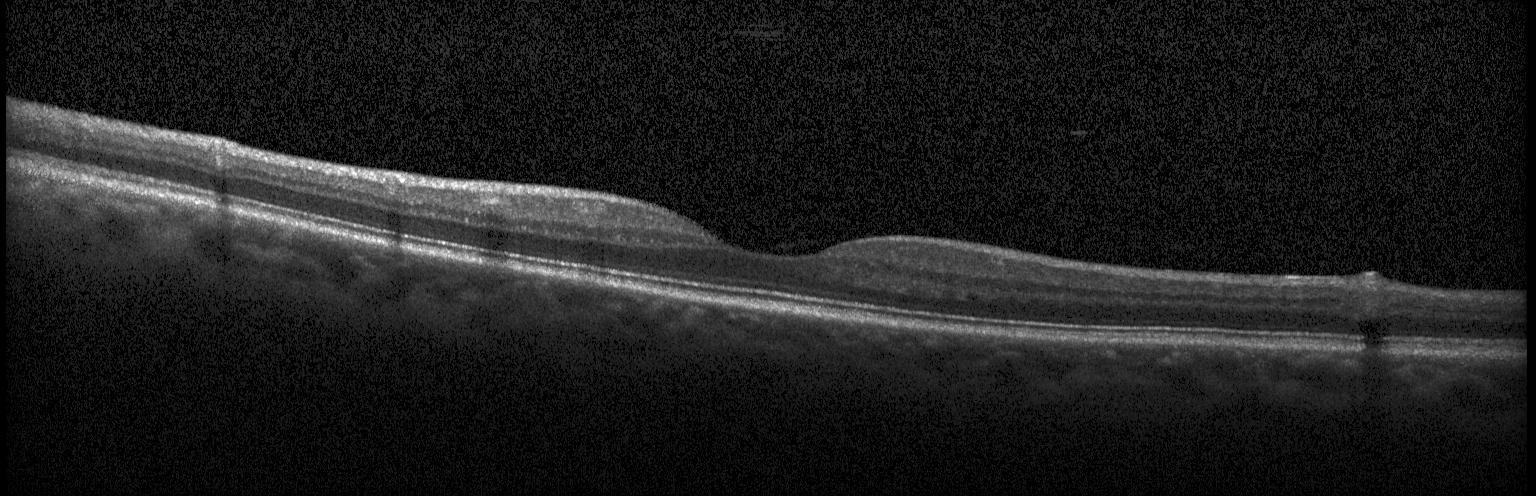 Retinal OCT cross-section · through the macula · Heidelberg Spectralis OCT system · SD-OCT — Diagnosis: neither choroidal neovascularization, diabetic macular edema, nor drusen.